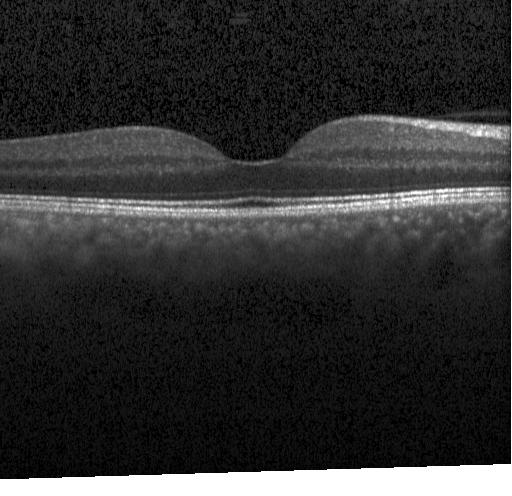

Acquired on a Heidelberg Spectralis, fovea-centered, OCT line scan — Finding: neither choroidal neovascularization, diabetic macular edema, nor drusen.